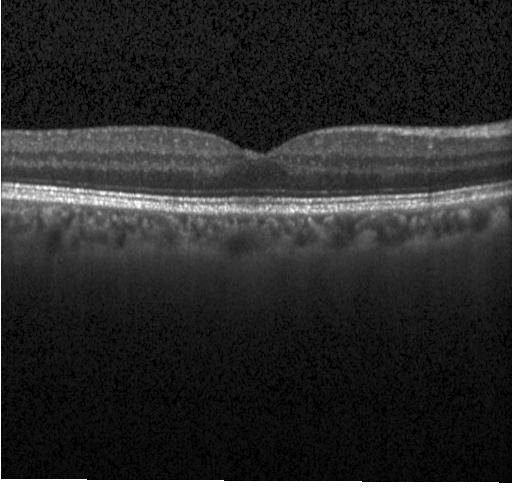
Impression: no evidence of choroidal neovascularization, diabetic macular edema, or drusen.